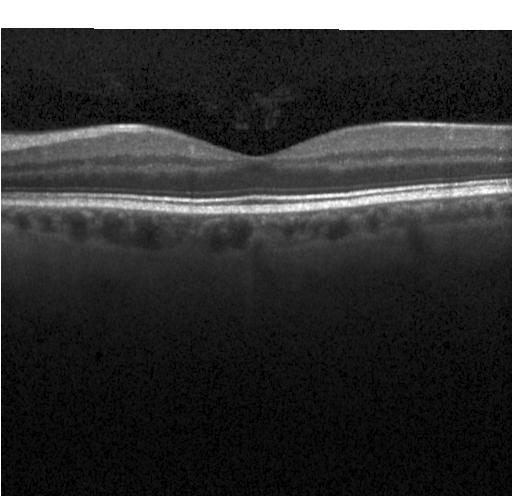

Dx: neither CNV, DME, nor drusen.